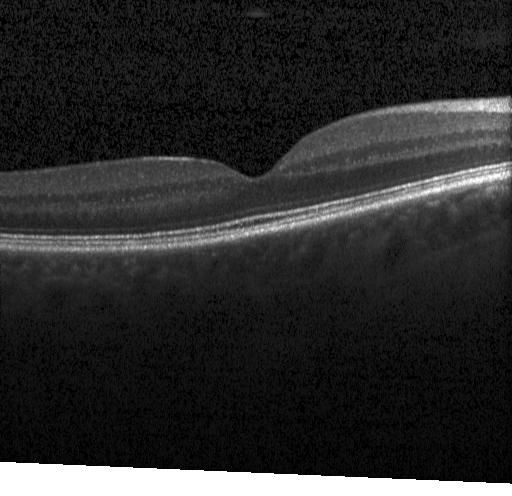
Spectral-domain optical coherence tomography, retinal OCT cross-section. Finding: neither choroidal neovascularization, diabetic macular edema, nor drusen.